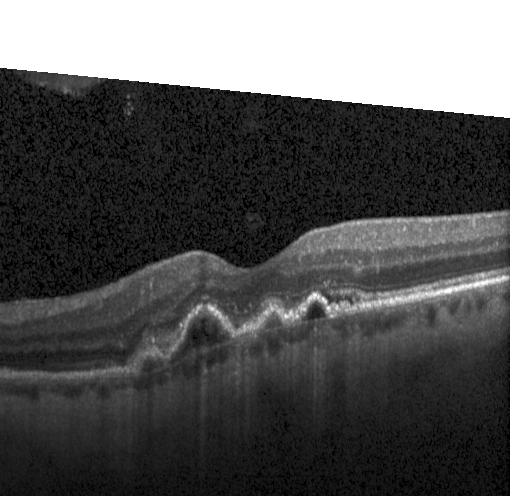

SD-OCT. OCT line scan. Through the macula. Instrument: Heidelberg Spectralis — Dx: a choroidal neovascular membrane.